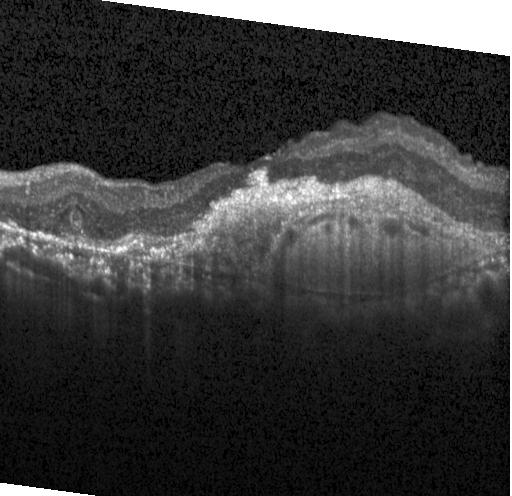 Macular OCT demonstrating choroidal neovascularization.